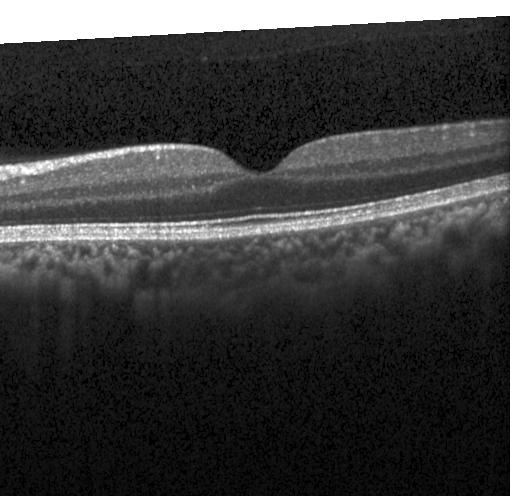
Fovea-centered, optical coherence tomography B-scan.
Impression: no choroidal neovascularization, diabetic macular edema, or drusen.